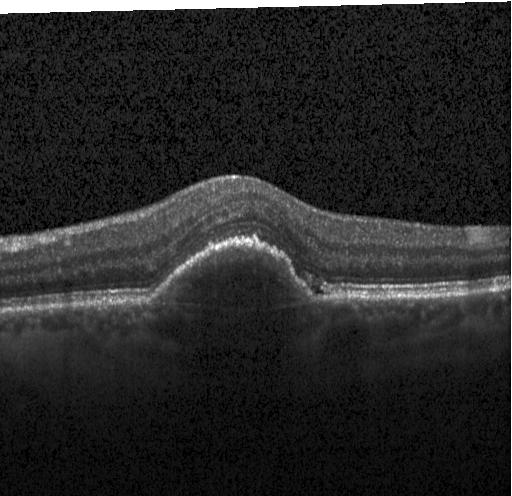
Retinal OCT B-scan · instrument: Heidelberg Spectralis · spectral-domain optical coherence tomography — This B-scan demonstrates a choroidal neovascular membrane.